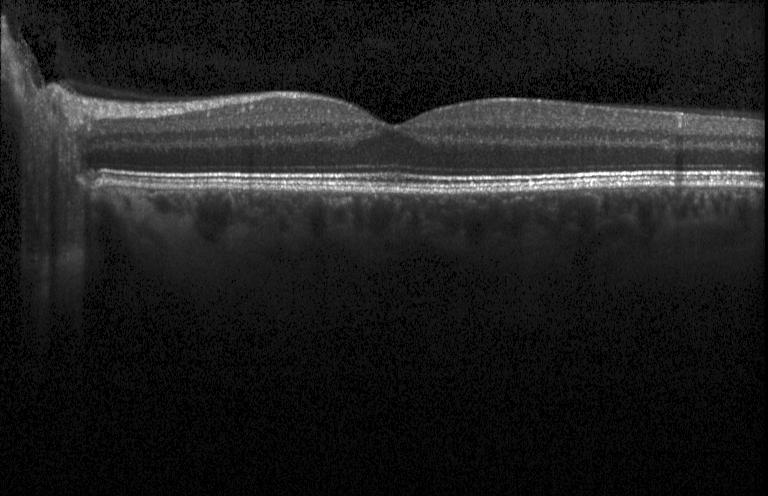
Dx: no choroidal neovascularization, no diabetic macular edema, and no drusen.